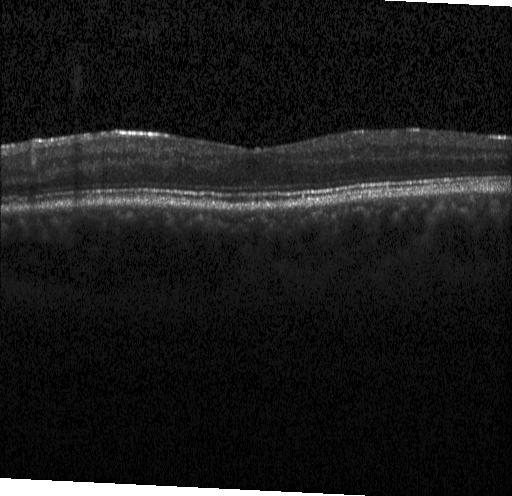 Spectral-domain OCT, optical coherence tomography scan
This B-scan demonstrates neither choroidal neovascularization, diabetic macular edema, nor drusen.